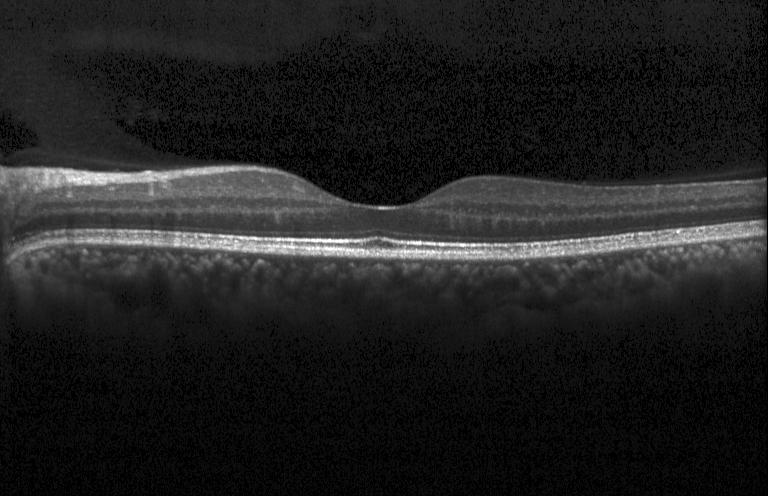 Spectral-domain OCT · optical coherence tomography scan
Impression: neither choroidal neovascularization, diabetic macular edema, nor drusen.